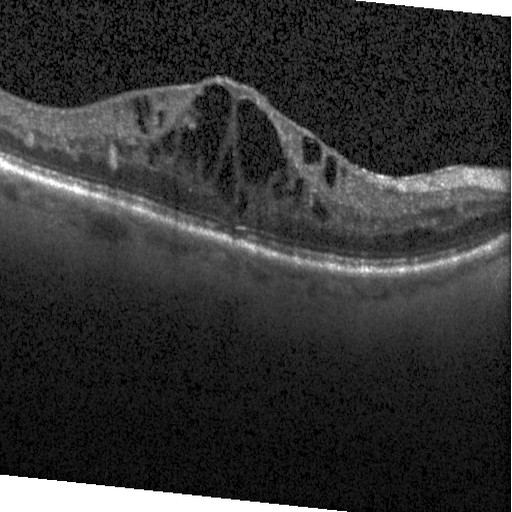

Impression: DME.